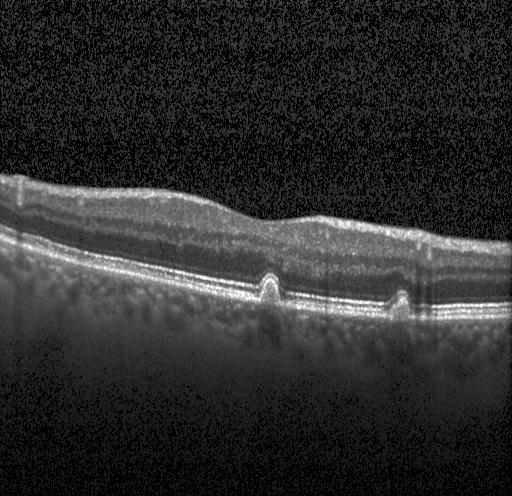
Retinal OCT B-scan.
Impression: multiple drusen.